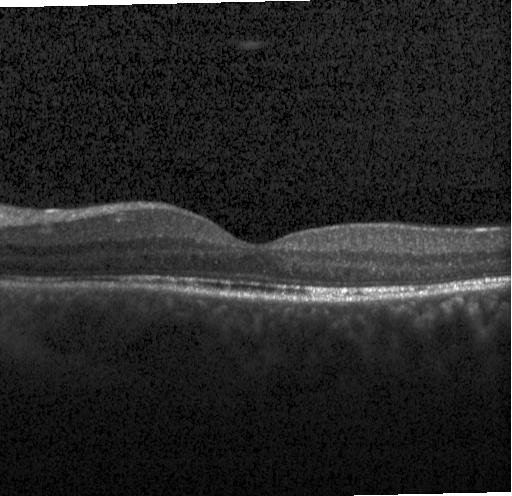

OCT B-scan; spectral-domain OCT; centered on the fovea — Macular OCT: neither choroidal neovascularization, diabetic macular edema, nor drusen.